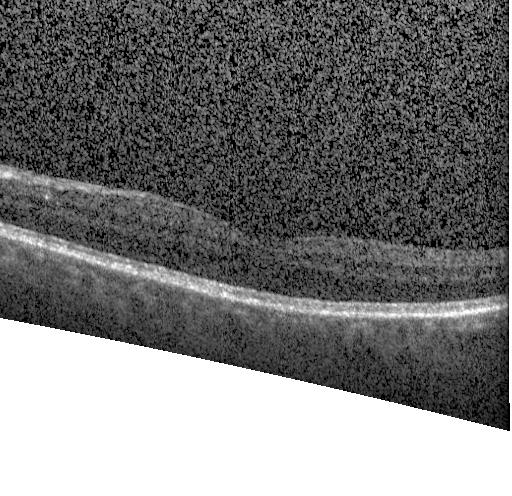 SD-OCT; optical coherence tomography B-scan; acquired on a Heidelberg Spectralis.
Finding: neither choroidal neovascularization, diabetic macular edema, nor drusen.